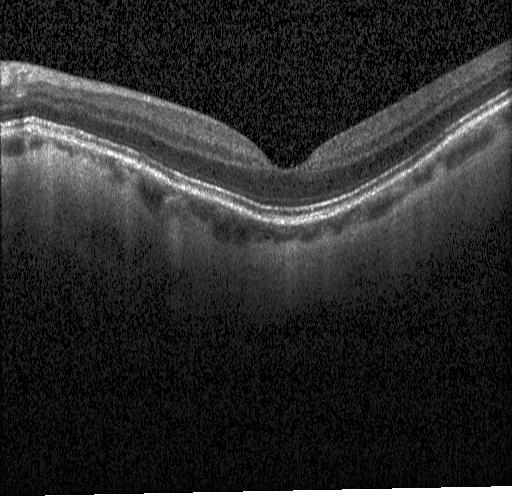
Retinal OCT cross-section. The scan shows no CNV, DME, or drusen.